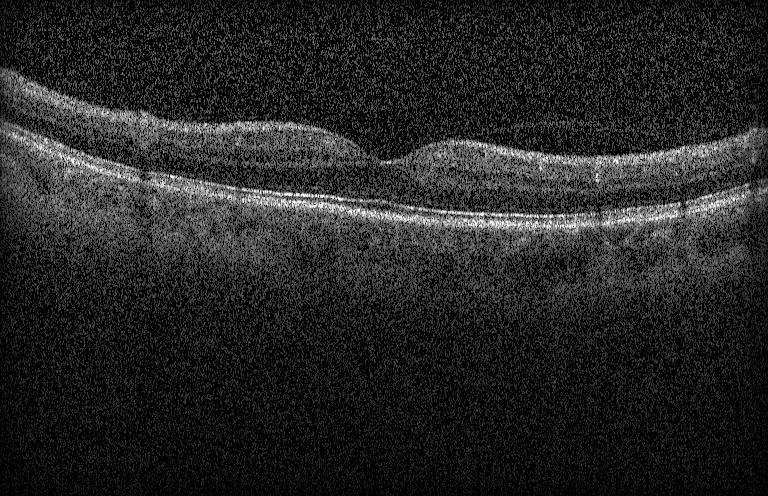

Macular scan · optical coherence tomography scan. Macular OCT: no evidence of CNV, DME, or drusen.